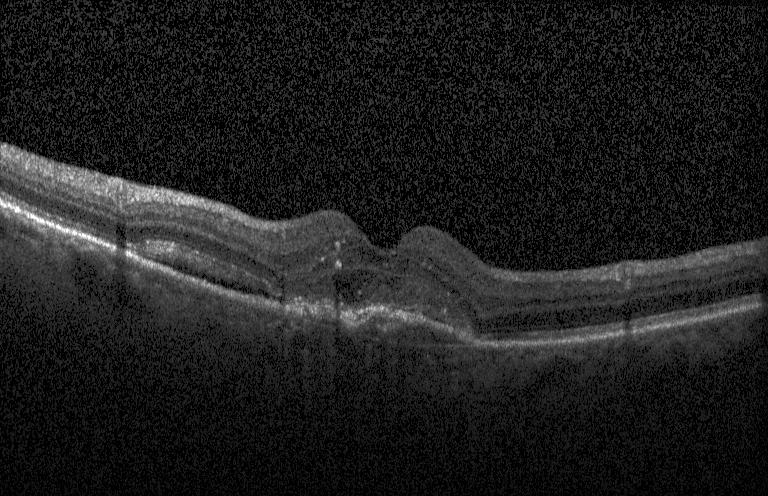

OCT finding: choroidal neovascularization (CNV).